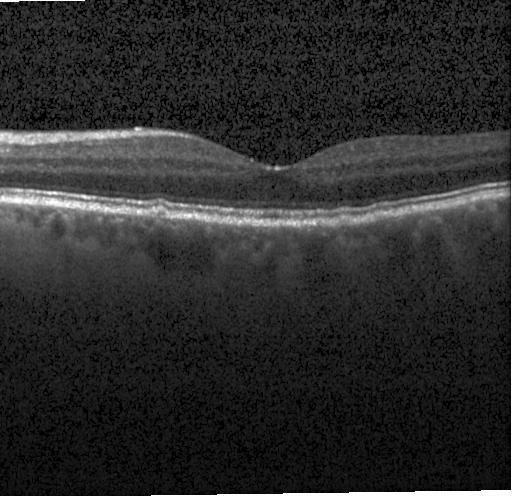
Assessment: drusen.